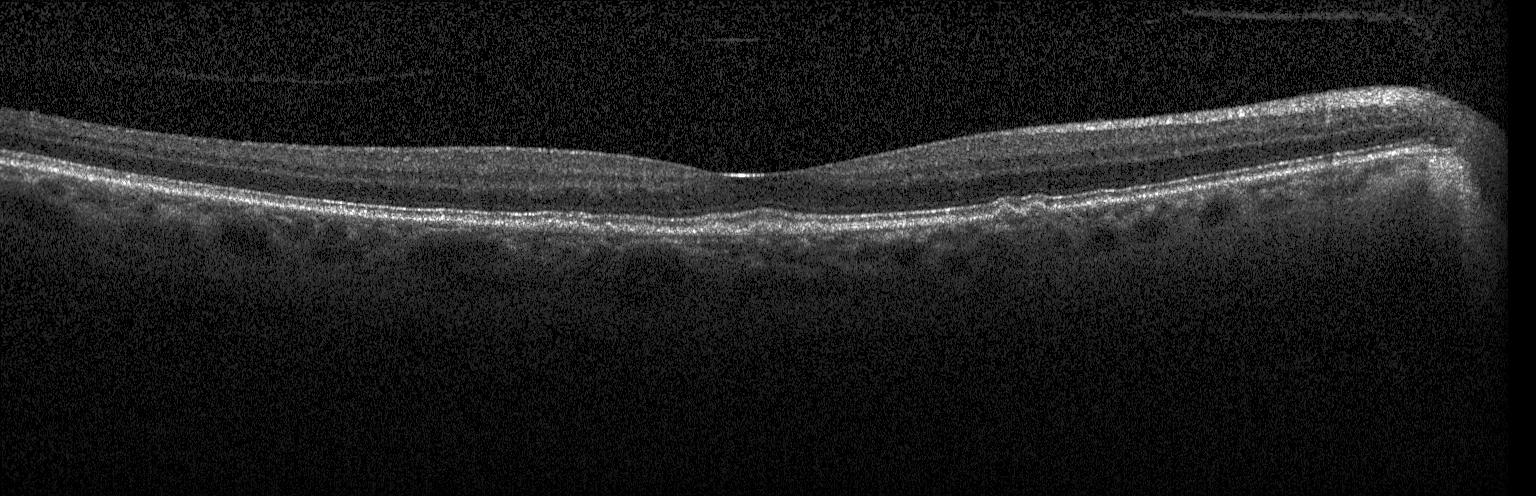

Assessment: sub-RPE drusenoid deposits.